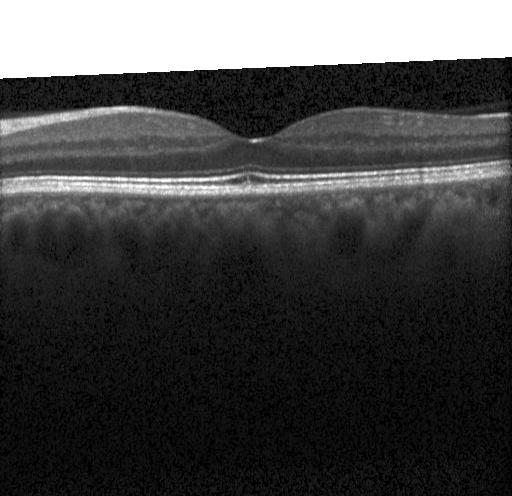

Retinal OCT B-scan · horizontal scan through the fovea. Macular OCT: no choroidal neovascularization, diabetic macular edema, or drusen.